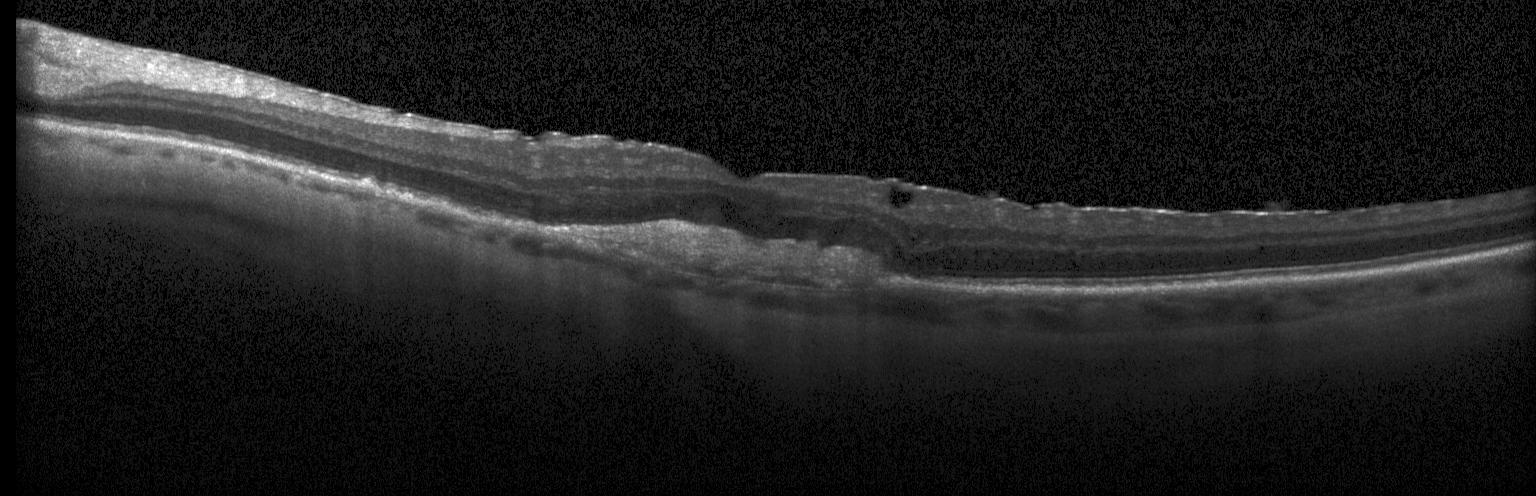 Instrument: Heidelberg Spectralis, retinal OCT B-scan
Assessment: a choroidal neovascular membrane.